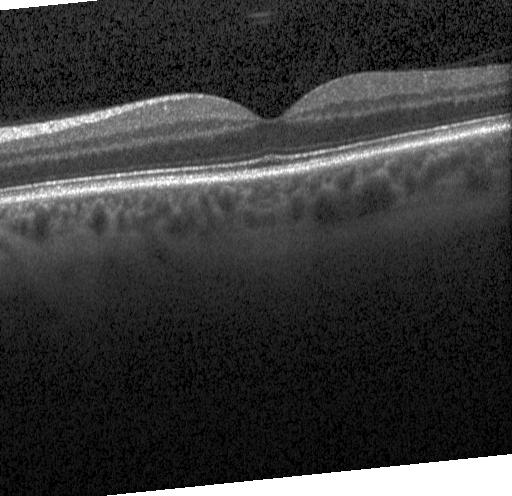 The scan shows no choroidal neovascularization, no diabetic macular edema, and no drusen.